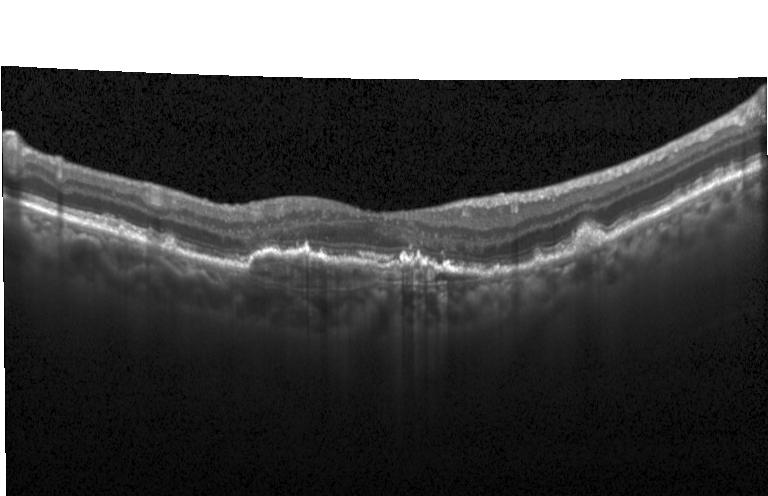

CNV.